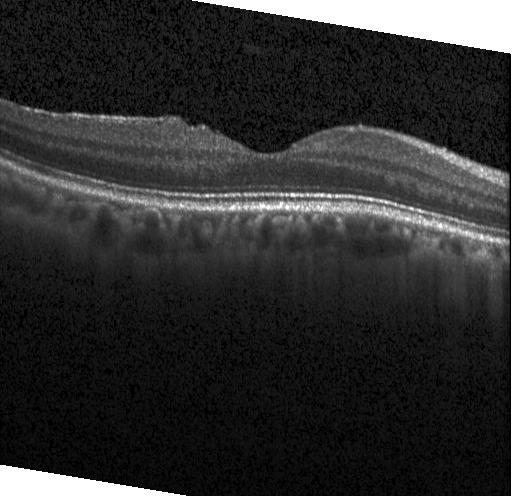 Retinal OCT cross-section, Heidelberg Spectralis OCT system — Macular OCT: no choroidal neovascularization, diabetic macular edema, or drusen.